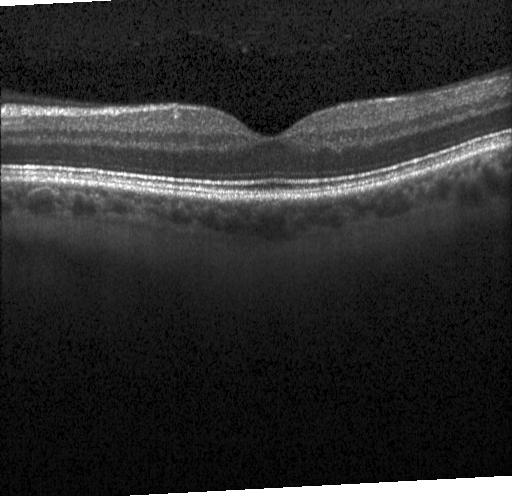 Instrument: Heidelberg Spectralis · optical coherence tomography B-scan · fovea-centered — Finding: no CNV, DME, or drusen.